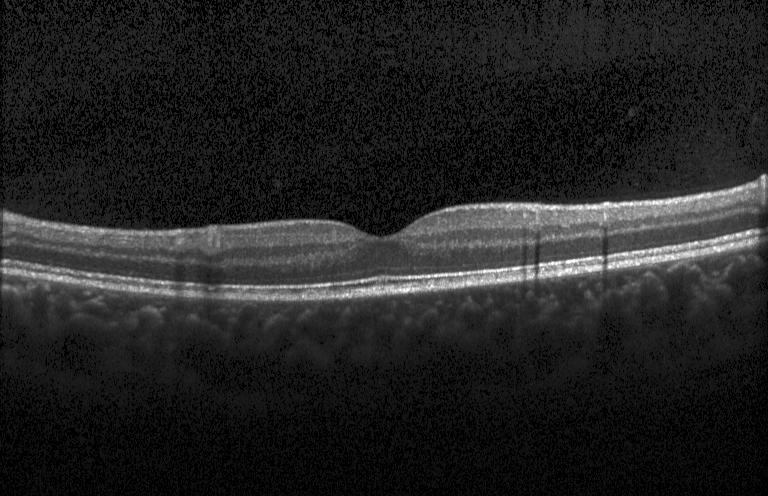
OCT B-scan, Heidelberg Spectralis OCT system, through the macula, spectral-domain OCT.
Finding: no choroidal neovascularization, diabetic macular edema, or drusen.